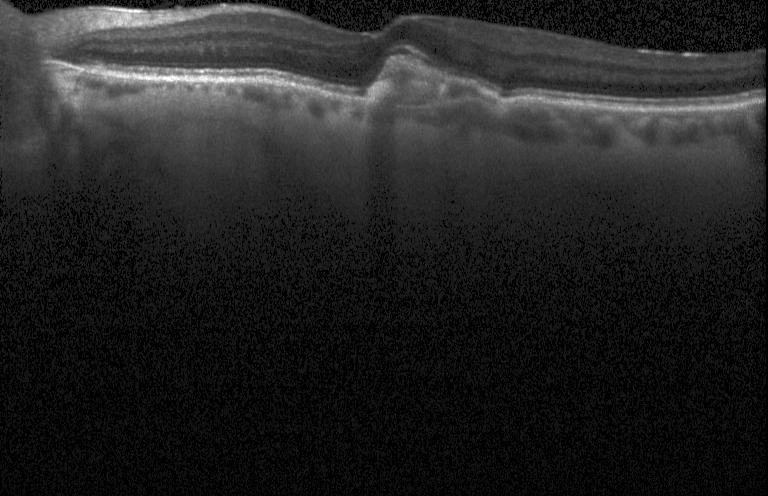

Centered on the fovea, spectral-domain OCT, OCT line scan, Heidelberg Spectralis — Impression: CNV.